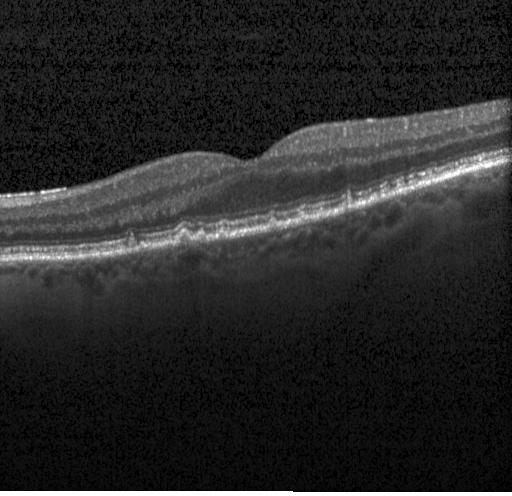
Diagnosis: multiple drusen.